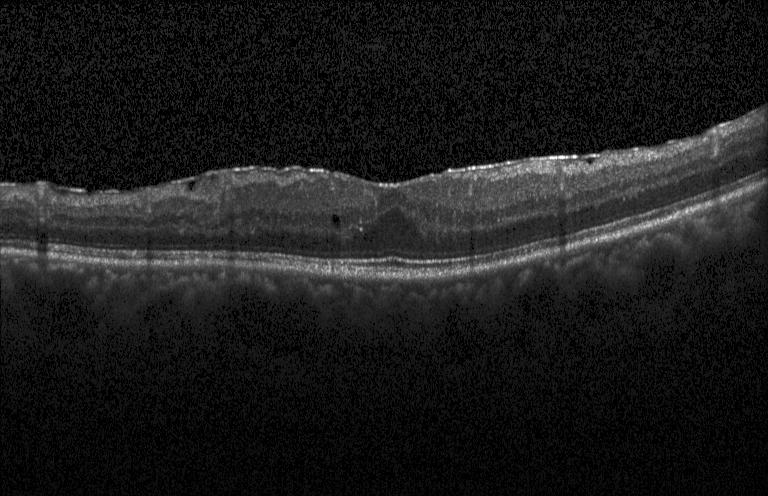

The scan shows diabetic macular edema.